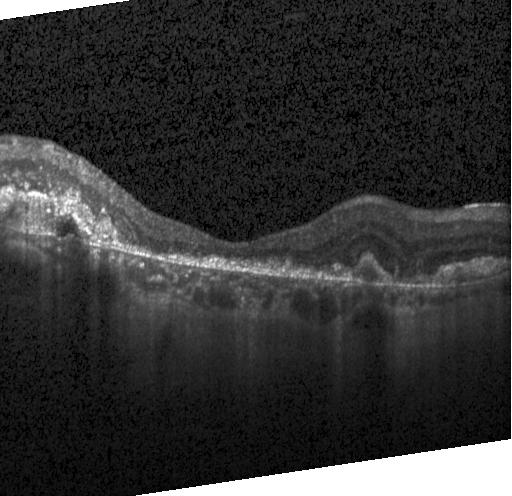 OCT line scan, horizontal scan through the fovea, SD-OCT.
Finding: choroidal neovascularization (CNV).